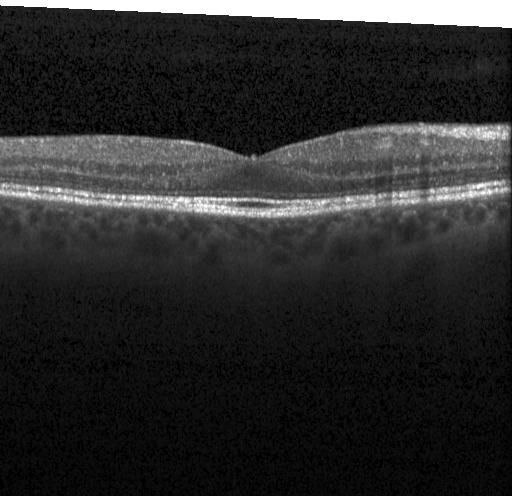
OCT line scan; acquired on a Heidelberg Spectralis
No choroidal neovascularization, no diabetic macular edema, and no drusen.